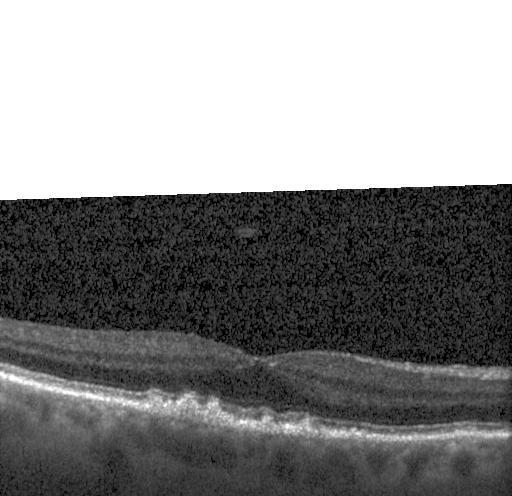
Spectral-domain optical coherence tomography, retinal OCT cross-section, instrument: Heidelberg Spectralis, macular scan. This B-scan demonstrates multiple drusen.